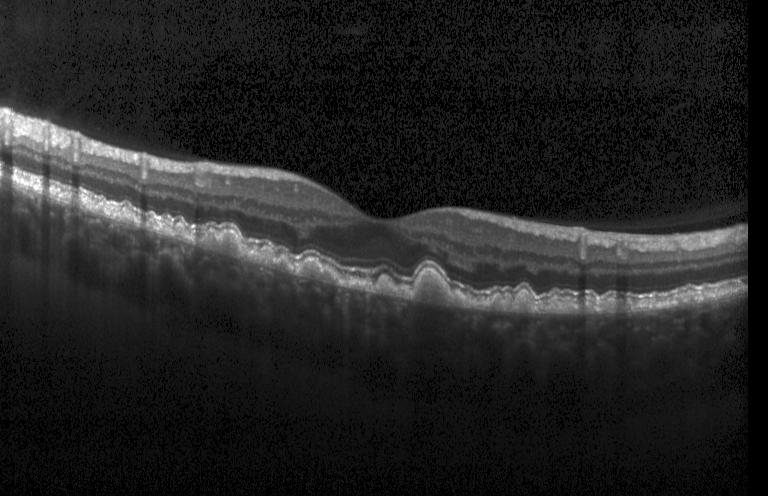
SD-OCT. Acquired on a Heidelberg Spectralis. OCT line scan.
Sub-RPE drusenoid deposits.